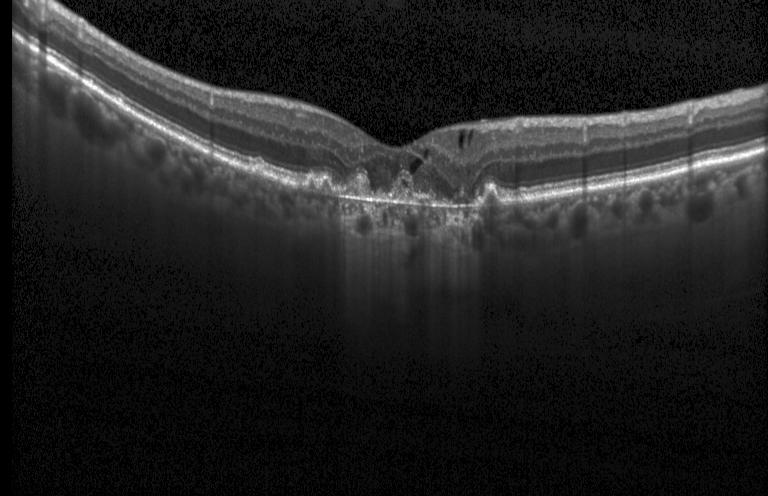

Centered on the fovea. SD-OCT. OCT line scan. Acquired on a Heidelberg Spectralis. Diagnosis: a choroidal neovascular membrane.